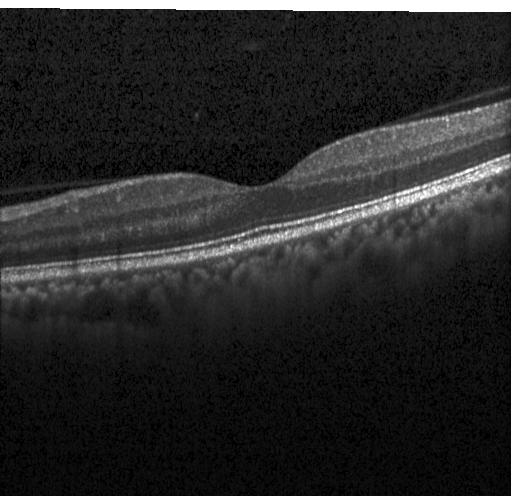
Retinal OCT cross-section; Heidelberg Spectralis; spectral-domain OCT. Diagnosis: no choroidal neovascularization, diabetic macular edema, or drusen.